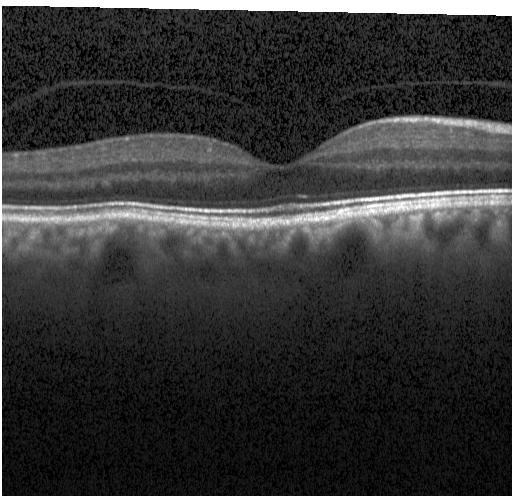 Diagnosis: no evidence of CNV, DME, or drusen.